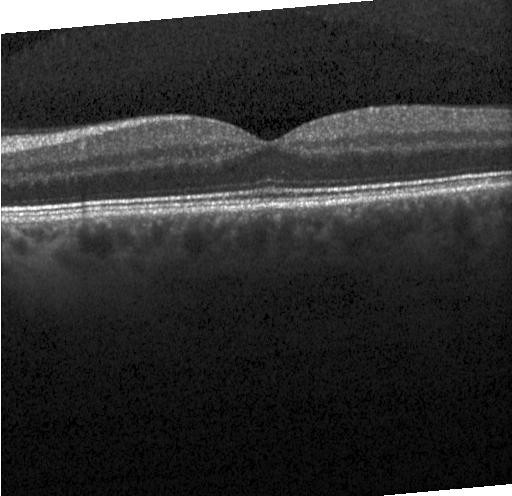
OCT B-scan · fovea-centered · instrument: Heidelberg Spectralis · spectral-domain optical coherence tomography
Dx: no evidence of CNV, DME, or drusen.